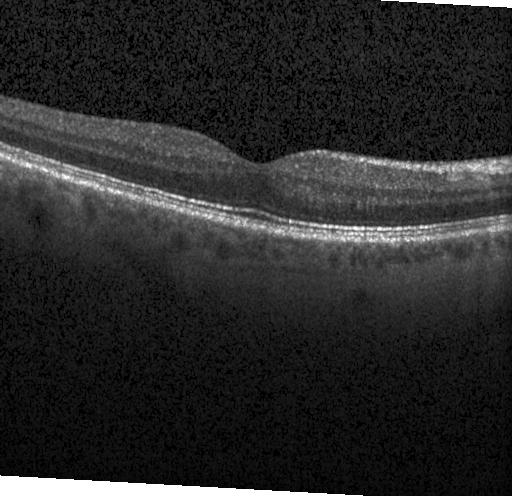 Heidelberg Spectralis OCT system. Retinal OCT cross-section. Centered on the fovea.
Macular OCT: no evidence of choroidal neovascularization, diabetic macular edema, or drusen.